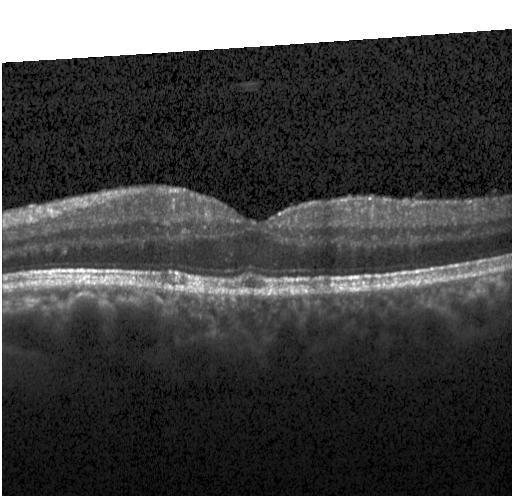
Heidelberg Spectralis OCT system, horizontal scan through the fovea, OCT B-scan. OCT finding: no evidence of choroidal neovascularization, diabetic macular edema, or drusen.